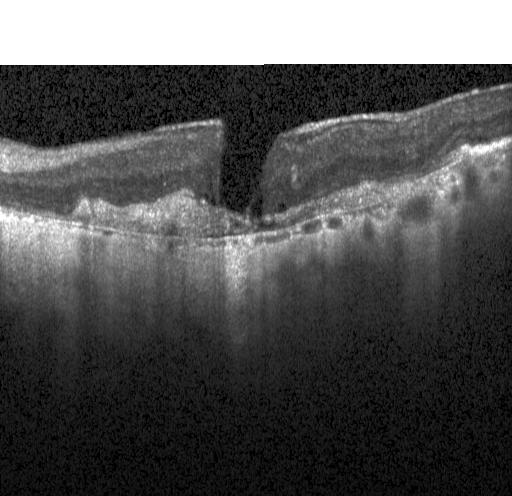

OCT scan showing a choroidal neovascular membrane.